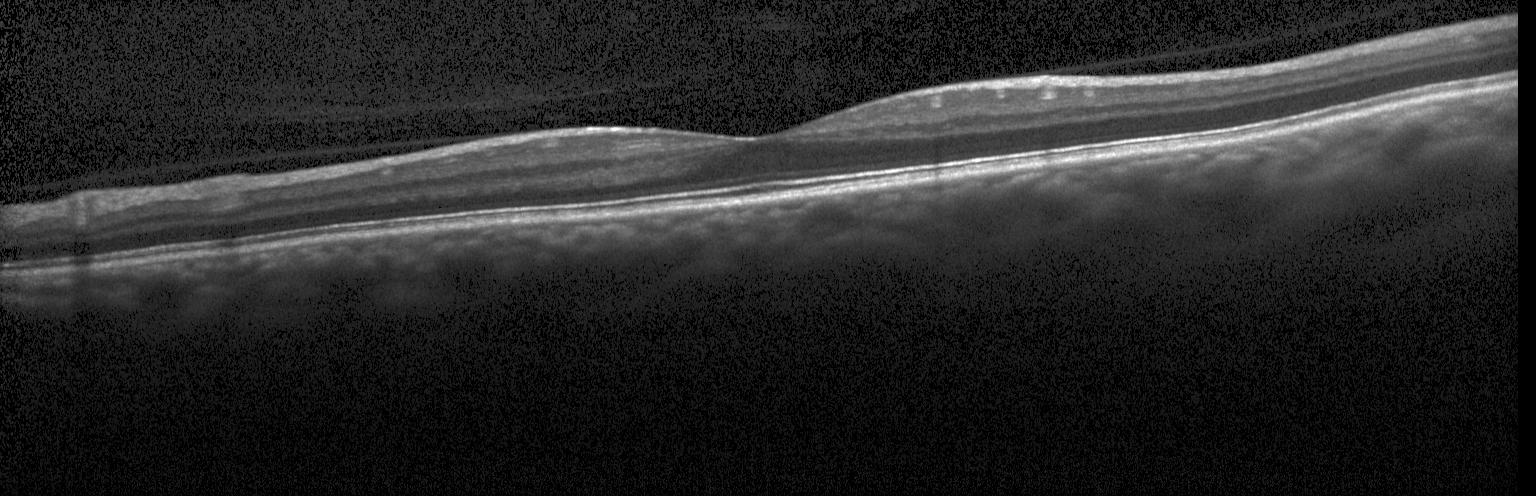

SD-OCT; horizontal scan through the fovea; OCT B-scan; Heidelberg Spectralis OCT system
Dx: neither CNV, DME, nor drusen.